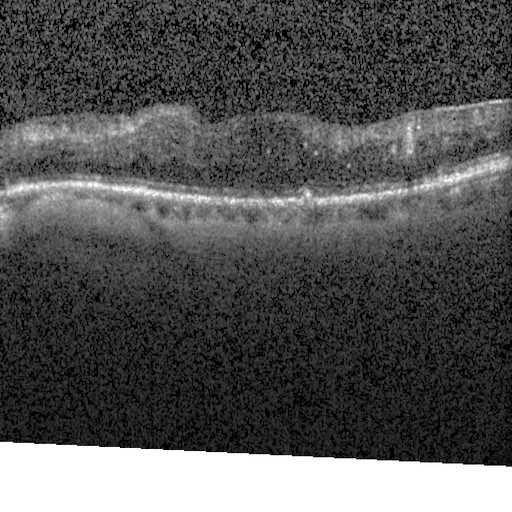 Heidelberg Spectralis. Centered on the fovea. Optical coherence tomography scan.
Impression: diabetic macular edema.